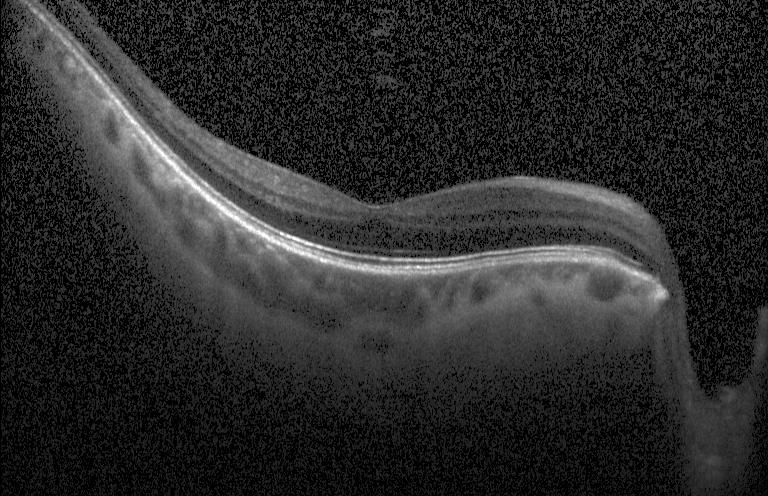 Retinal OCT B-scan. Assessment: no CNV, no DME, and no drusen.